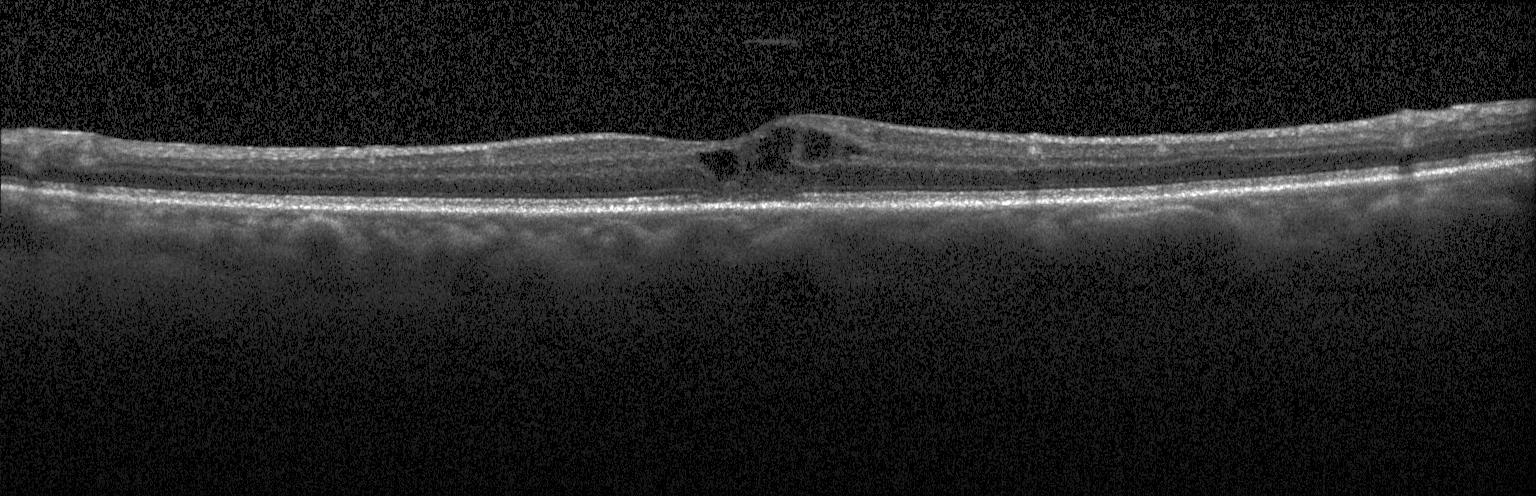 Impression: DME.